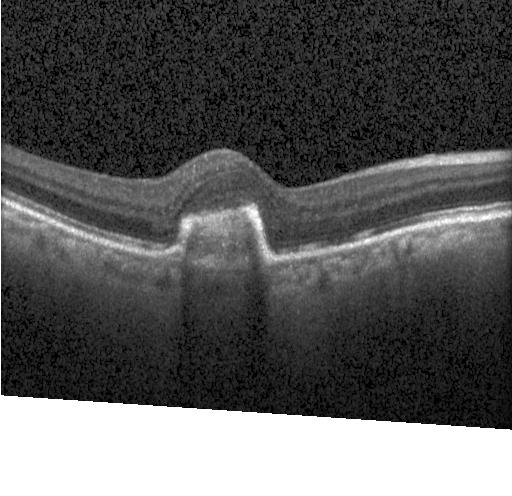 Fovea-centered, retinal OCT B-scan, spectral-domain optical coherence tomography
Macular OCT: choroidal neovascularization (CNV).